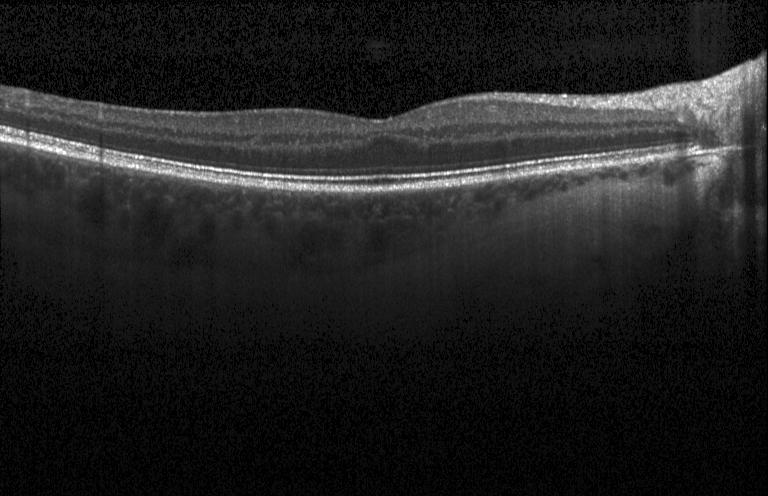 OCT B-scan. Neither CNV, DME, nor drusen.